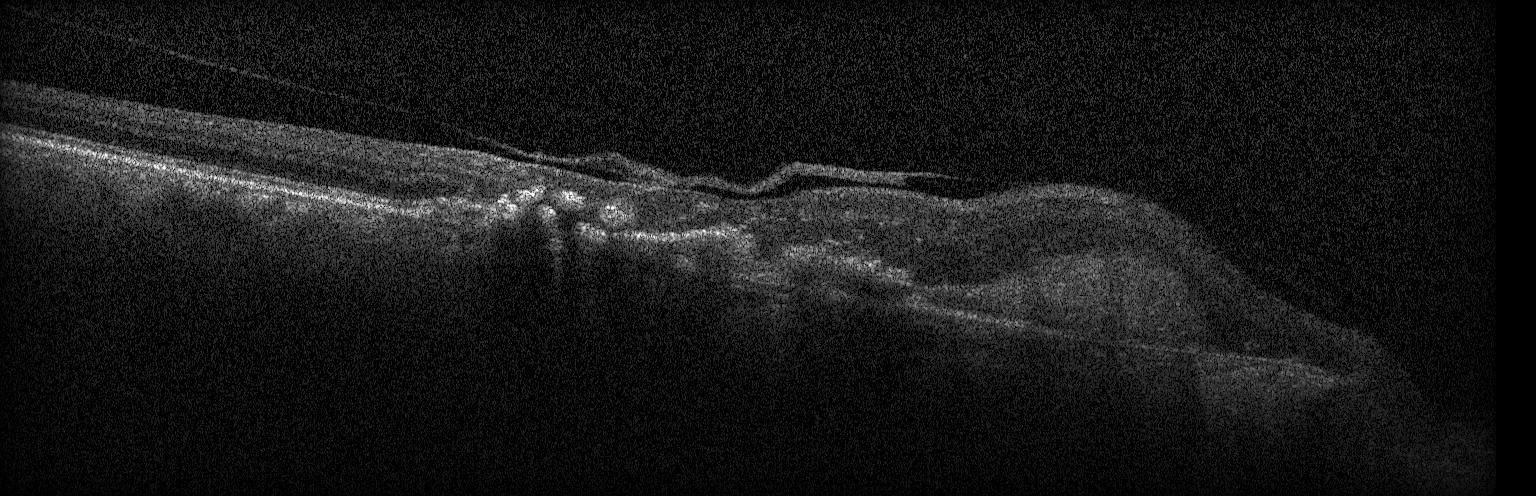 Optical coherence tomography scan.
CNV.